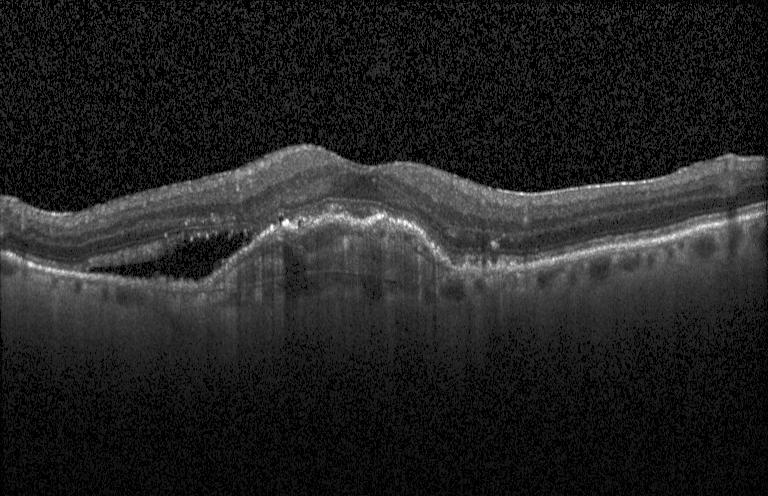 Impression: a choroidal neovascular membrane.